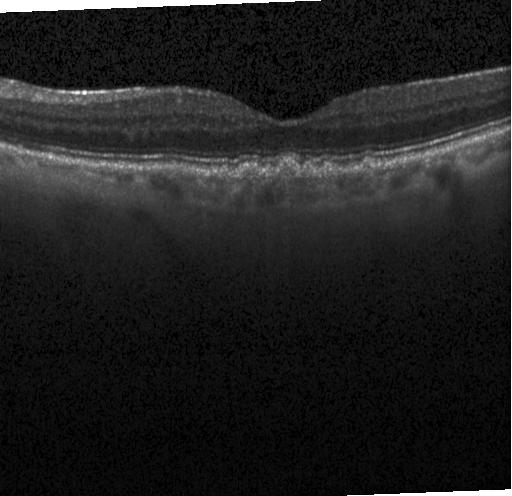 Spectral-domain optical coherence tomography; optical coherence tomography scan; through the macula
Diagnosis: sub-RPE drusenoid deposits.